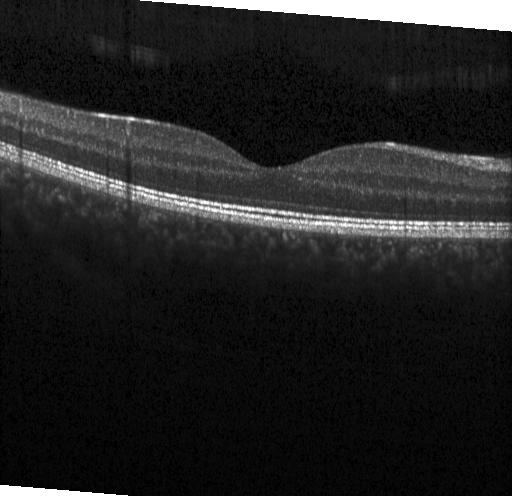
Retinal OCT cross-section. Assessment: no CNV, no DME, and no drusen.